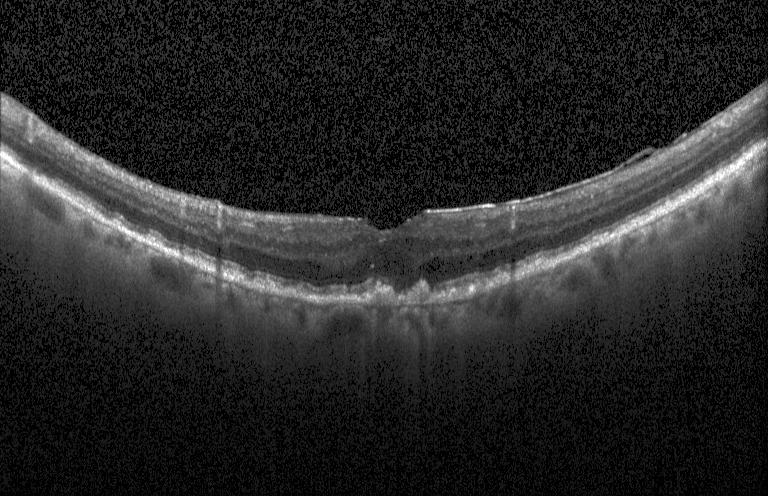

Retinal OCT cross-section
Diagnosis: drusen.